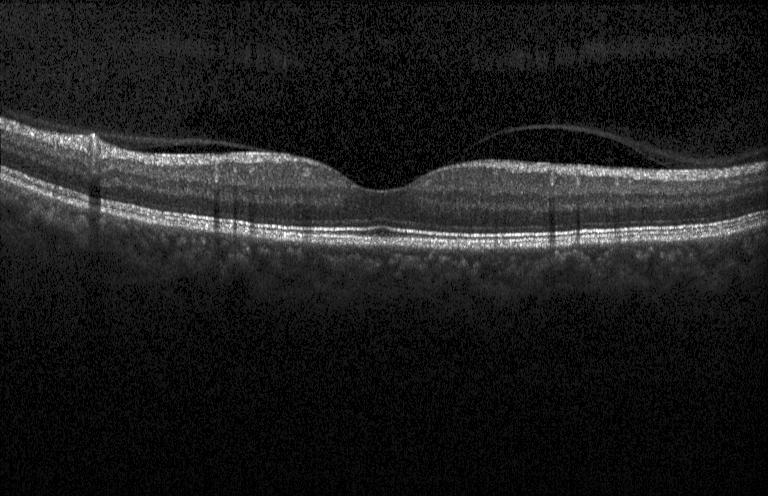

Retinal OCT cross-section · spectral-domain OCT · macular scan. The scan shows no CNV, DME, or drusen.